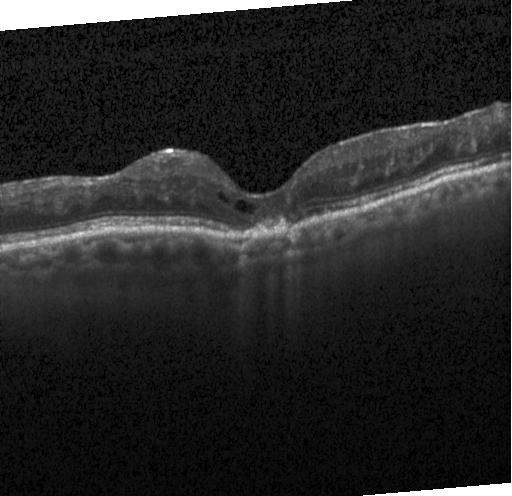

CNV.